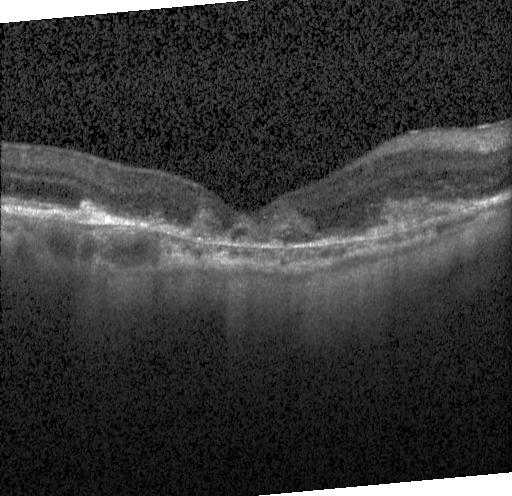

Macular scan · Heidelberg Spectralis OCT system · SD-OCT · retinal OCT cross-section.
The scan shows CNV.